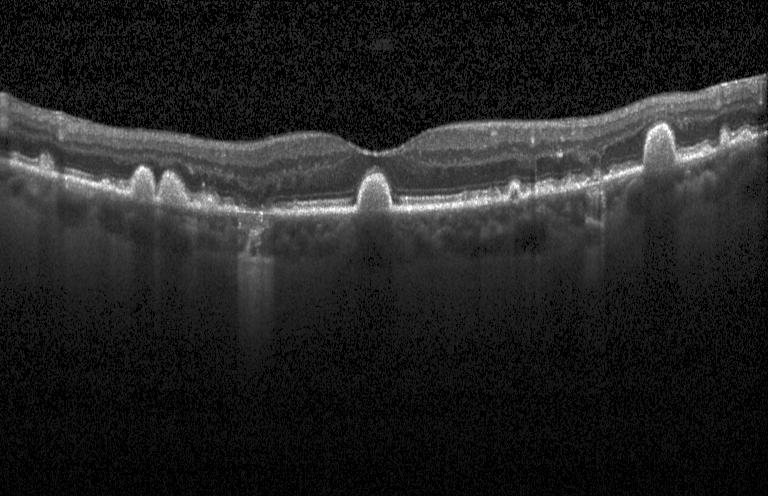

This B-scan demonstrates drusen.